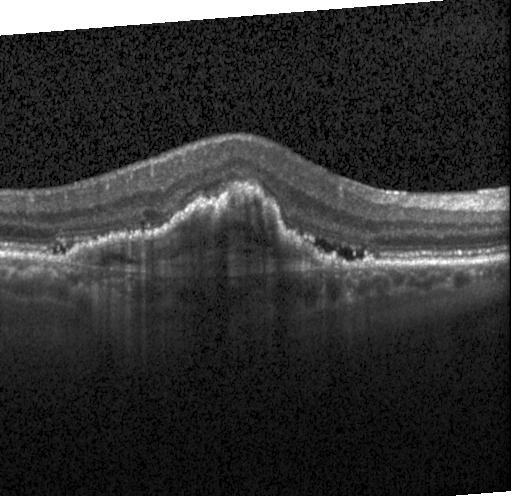 Heidelberg Spectralis. SD-OCT. Retinal OCT cross-section. Dx: a choroidal neovascular membrane.